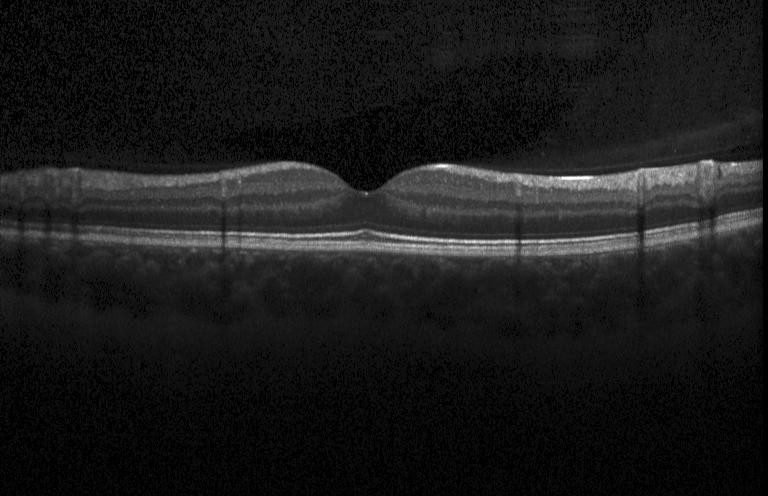 Diagnosis: no evidence of choroidal neovascularization, diabetic macular edema, or drusen.